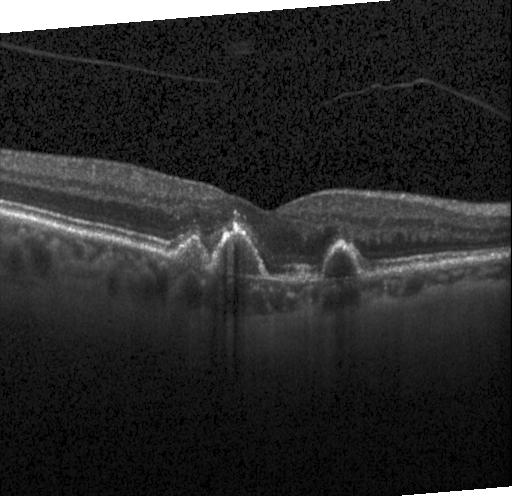

Heidelberg Spectralis; SD-OCT; macular scan; optical coherence tomography B-scan.
Impression: a choroidal neovascular membrane.